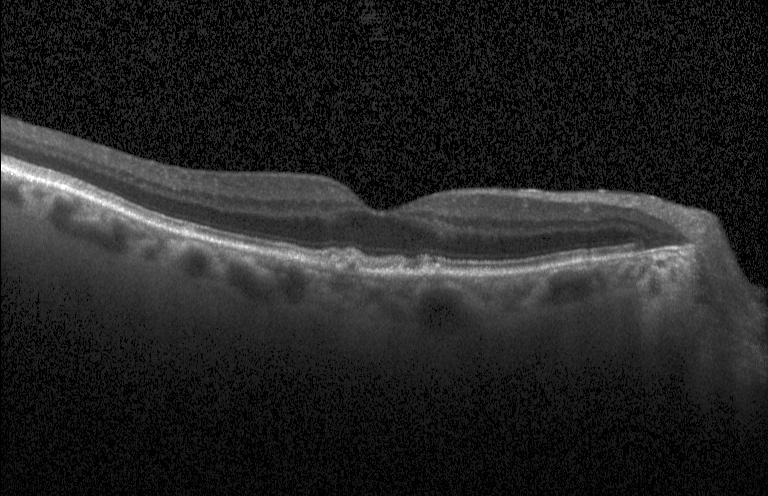 OCT B-scan showing drusen.